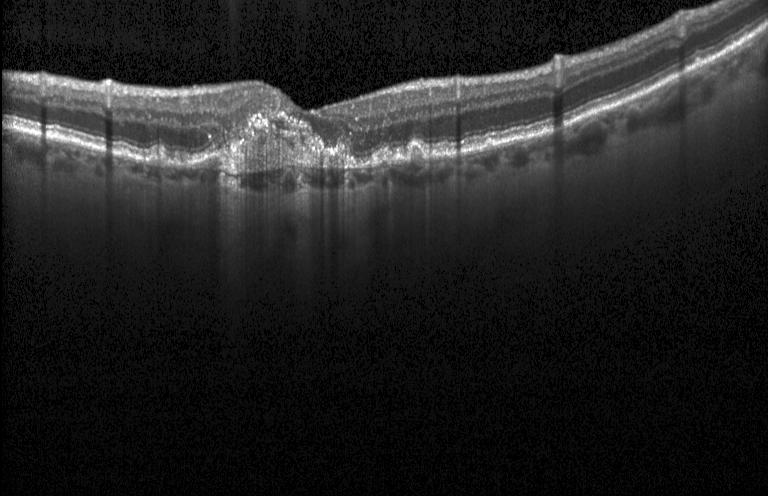 Spectral-domain OCT · OCT B-scan · instrument: Heidelberg Spectralis. Finding: choroidal neovascularization (CNV).